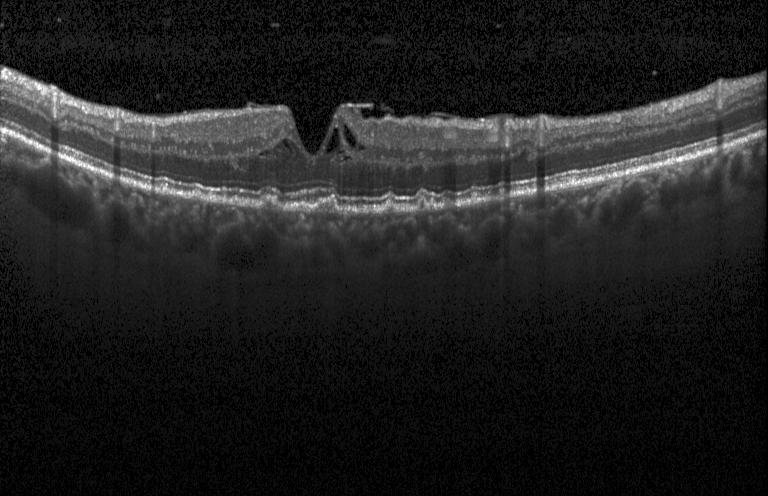

Assessment: multiple drusen.